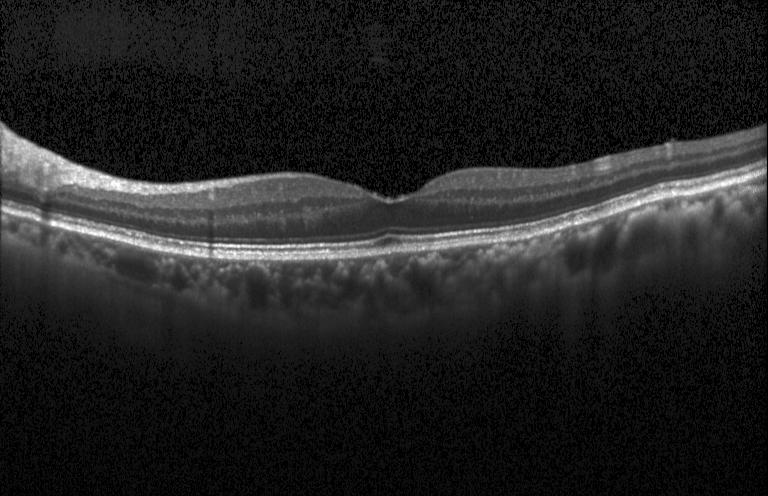

OCT finding: neither choroidal neovascularization, diabetic macular edema, nor drusen.